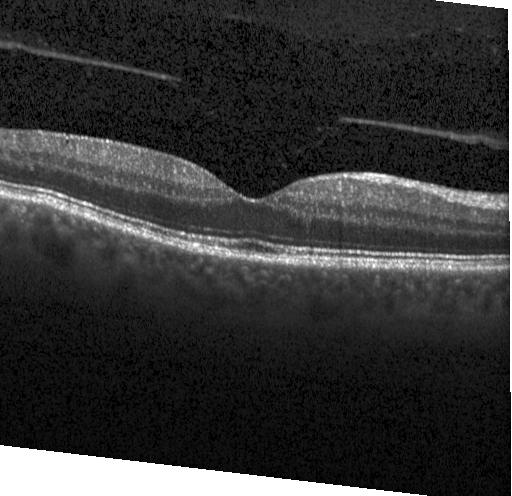 The scan shows no choroidal neovascularization, no diabetic macular edema, and no drusen.